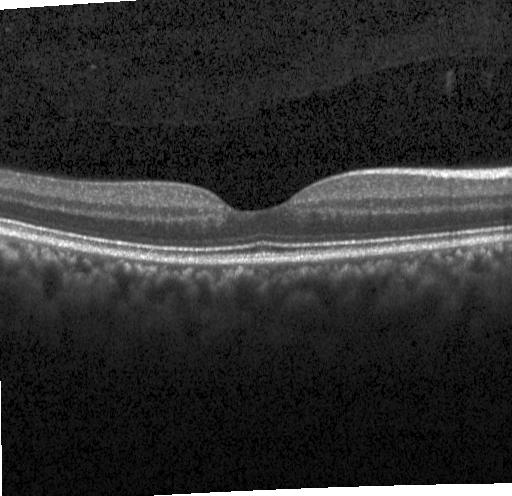
Spectral-domain OCT · OCT B-scan · horizontal scan through the fovea · Heidelberg Spectralis OCT system — Finding: neither choroidal neovascularization, diabetic macular edema, nor drusen.